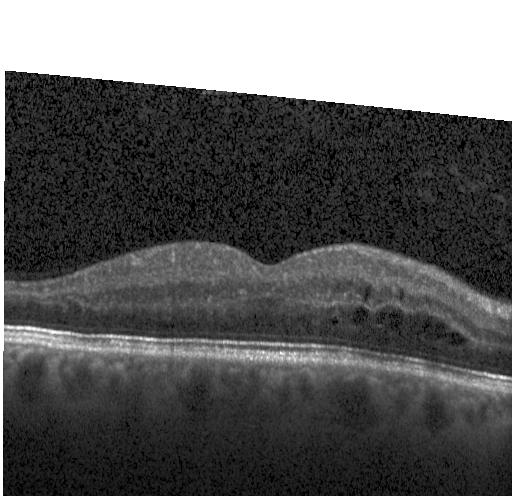
OCT line scan; spectral-domain OCT; horizontal scan through the fovea. The scan shows diabetic macular edema (DME).